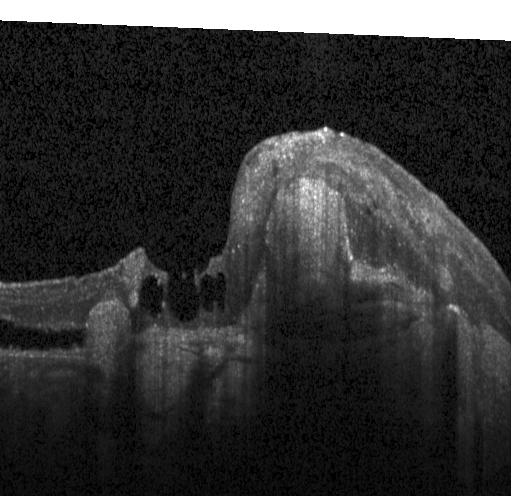 Finding: choroidal neovascularization.